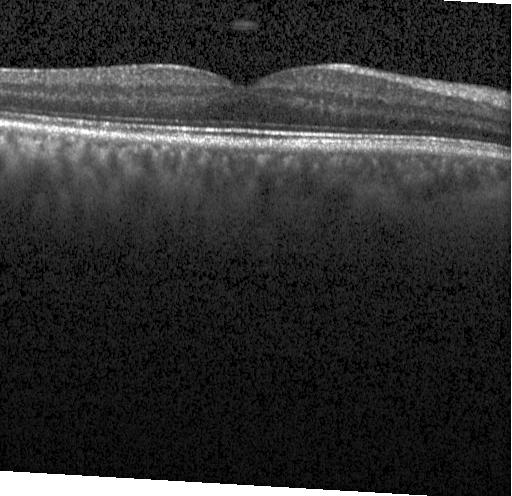
OCT B-scan. Instrument: Heidelberg Spectralis
Finding: no choroidal neovascularization, no diabetic macular edema, and no drusen.